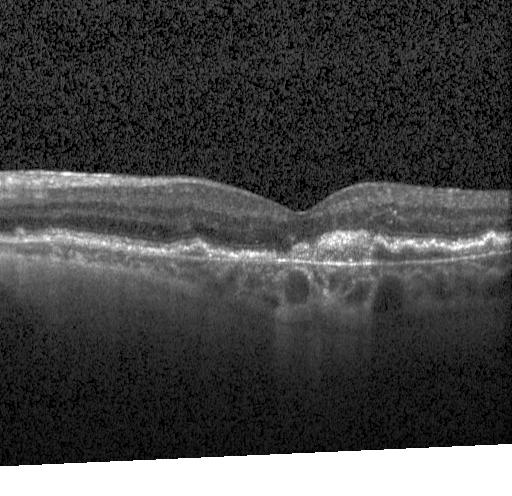
Acquired on a Heidelberg Spectralis. Retinal OCT B-scan.
Macular OCT: choroidal neovascularization.